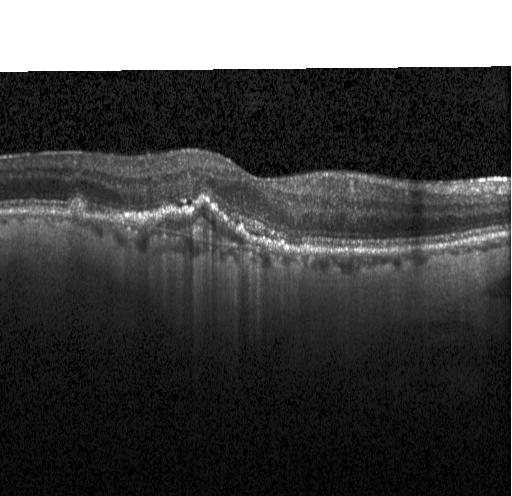

Optical coherence tomography B-scan; SD-OCT; Heidelberg Spectralis OCT system
Dx: CNV.